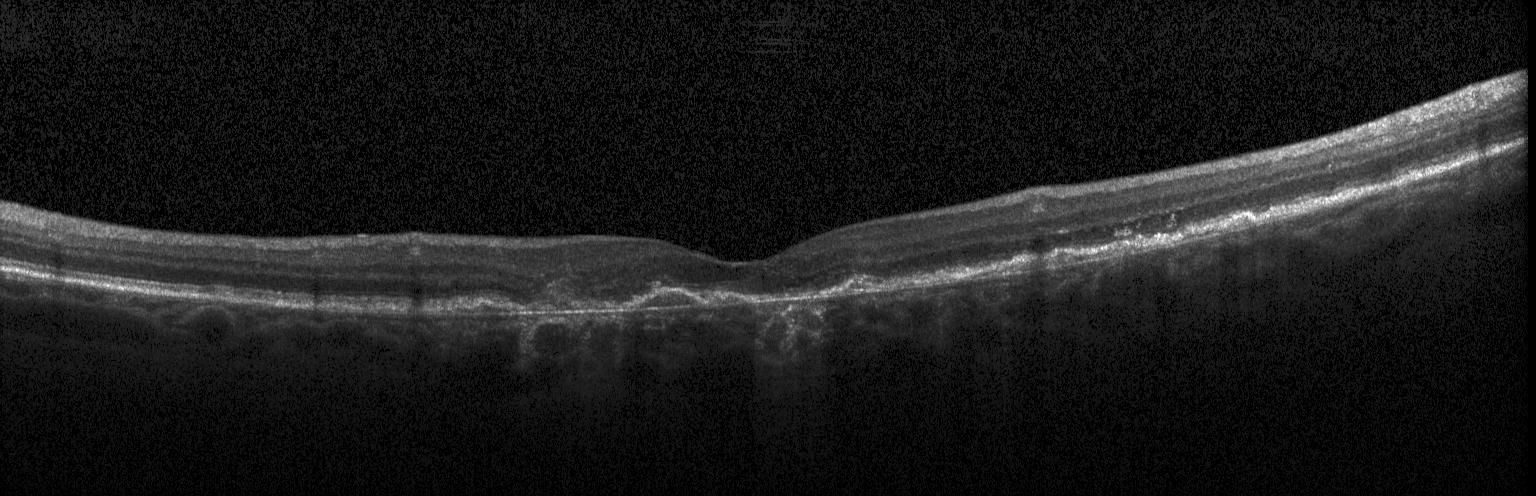
OCT B-scan; macular scan; Heidelberg Spectralis OCT system
Diagnosis: a choroidal neovascular membrane.